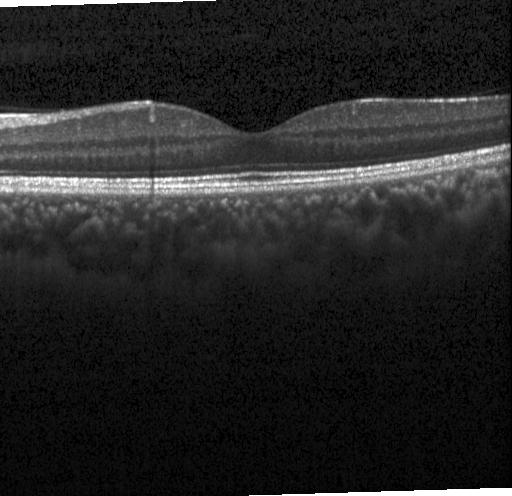
Heidelberg Spectralis · macular scan · OCT line scan. The scan shows no CNV, no DME, and no drusen.